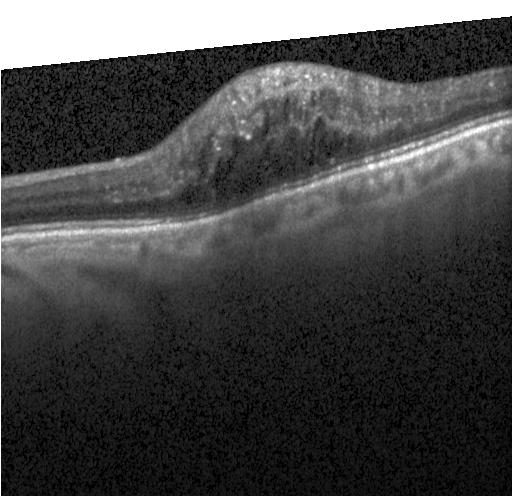 Macular OCT: diabetic macular edema (DME).